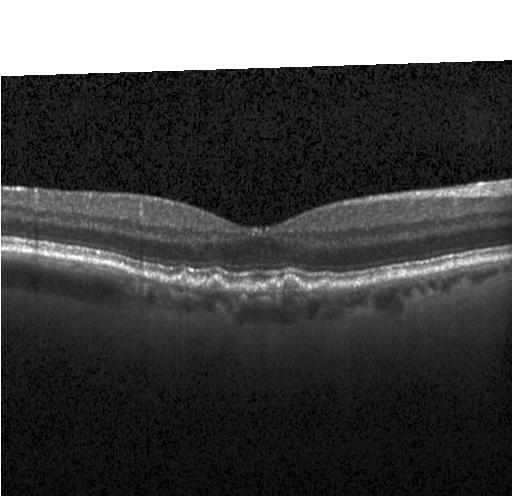
Retinal OCT B-scan — The scan shows drusen.